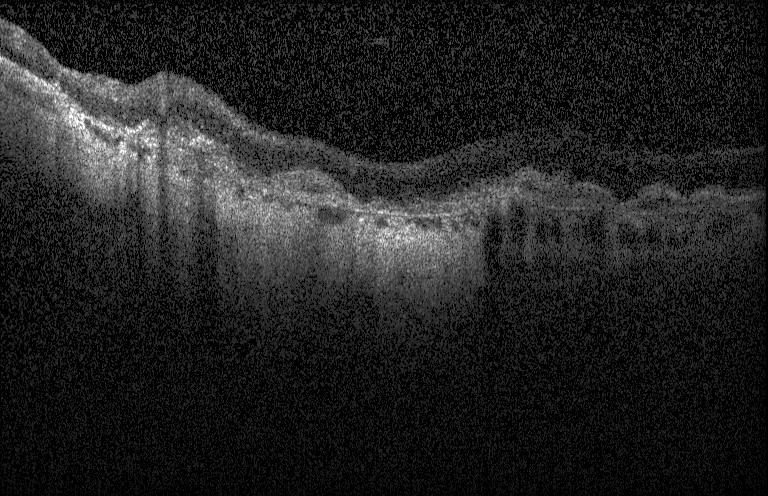
Macular scan; OCT line scan. Impression: choroidal neovascularization (CNV).